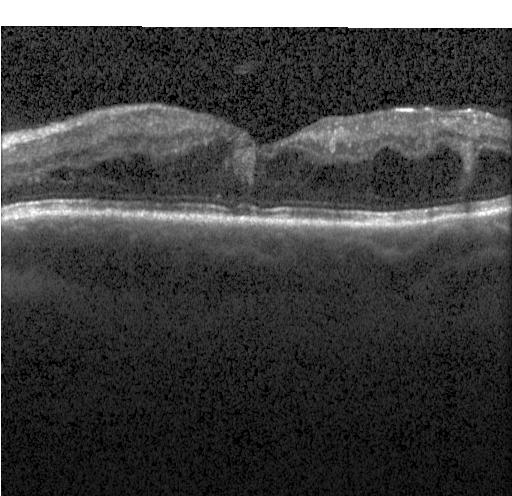 Dx: diabetic macular edema.